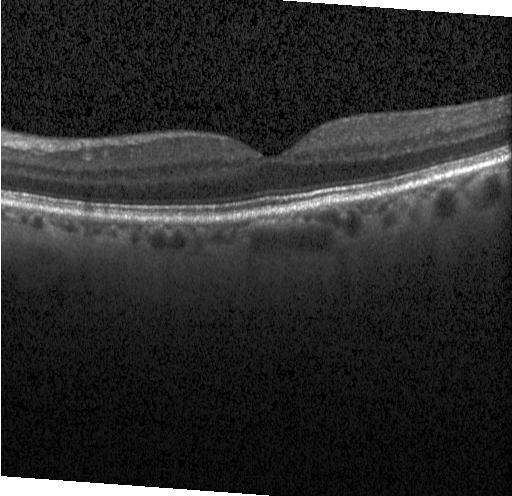
Finding: neither choroidal neovascularization, diabetic macular edema, nor drusen.